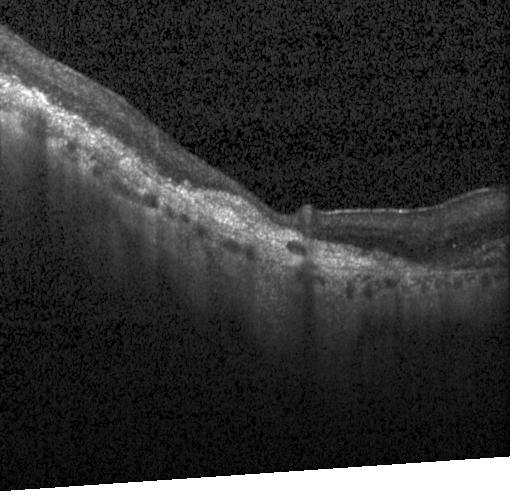 Retinal OCT B-scan · Heidelberg Spectralis OCT system. Diagnosis: a choroidal neovascular membrane.